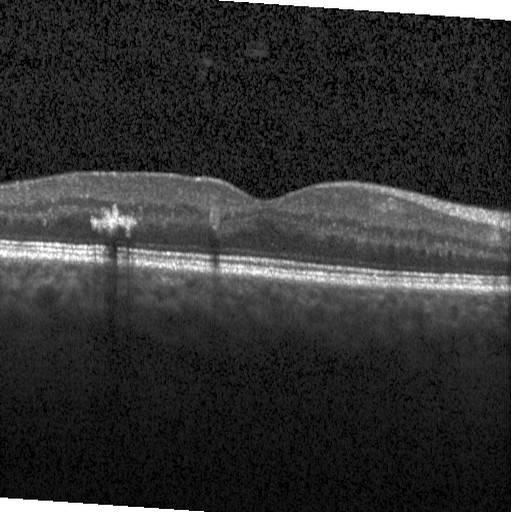 Instrument: Heidelberg Spectralis. Retinal OCT cross-section. Spectral-domain optical coherence tomography. Macular scan
The scan shows diabetic macular edema (DME).